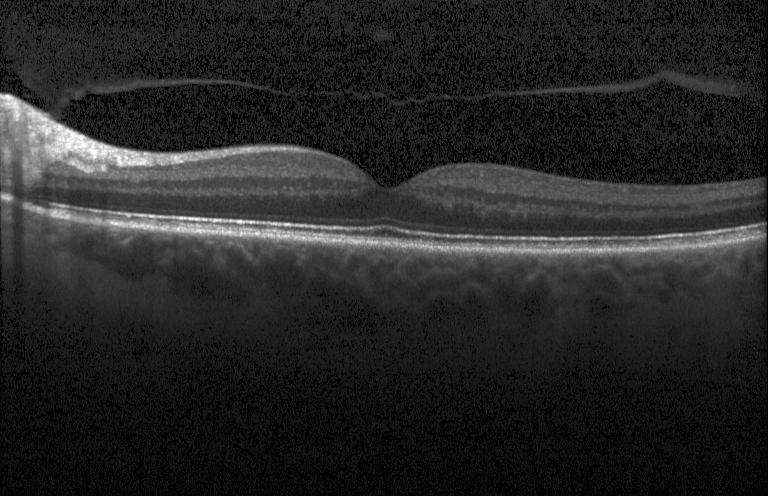

Optical coherence tomography scan. Diagnosis: no choroidal neovascularization, diabetic macular edema, or drusen.